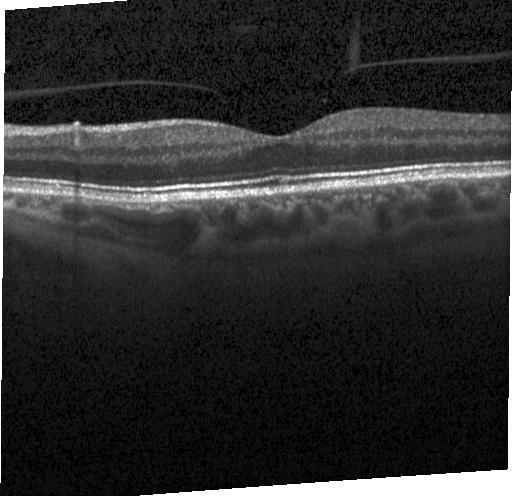
Spectral-domain OCT. Macular scan. Retinal OCT cross-section. Heidelberg Spectralis.
Finding: no CNV, DME, or drusen.